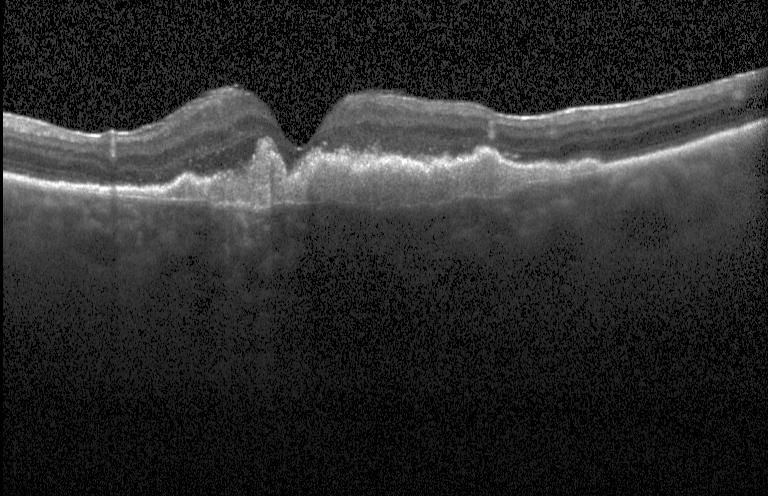 Finding: CNV.